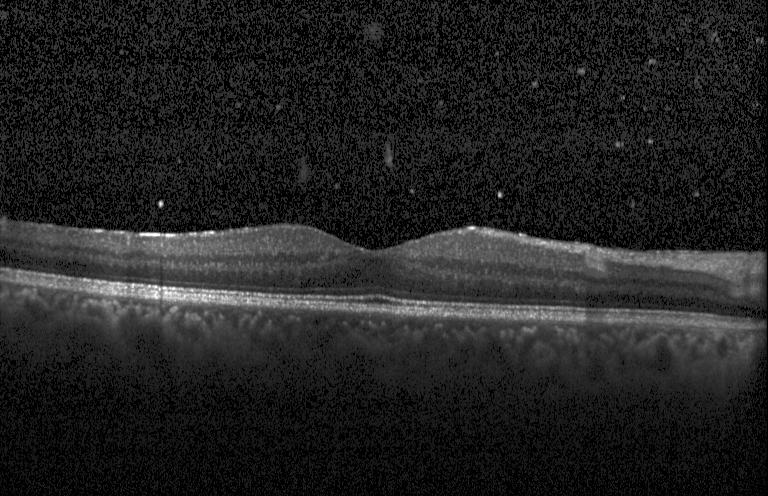 Through the macula · spectral-domain optical coherence tomography · optical coherence tomography B-scan
Finding: no choroidal neovascularization, diabetic macular edema, or drusen.